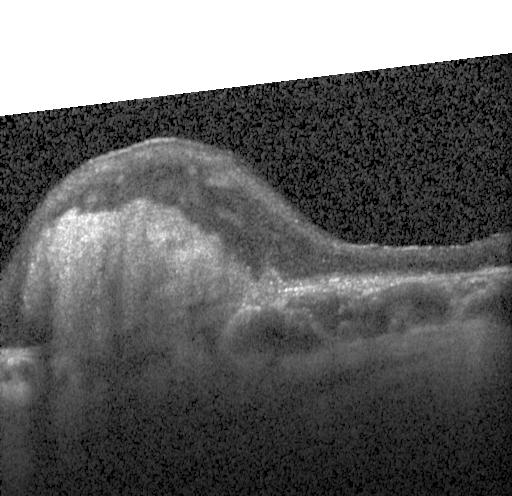
OCT scan showing a choroidal neovascular membrane.